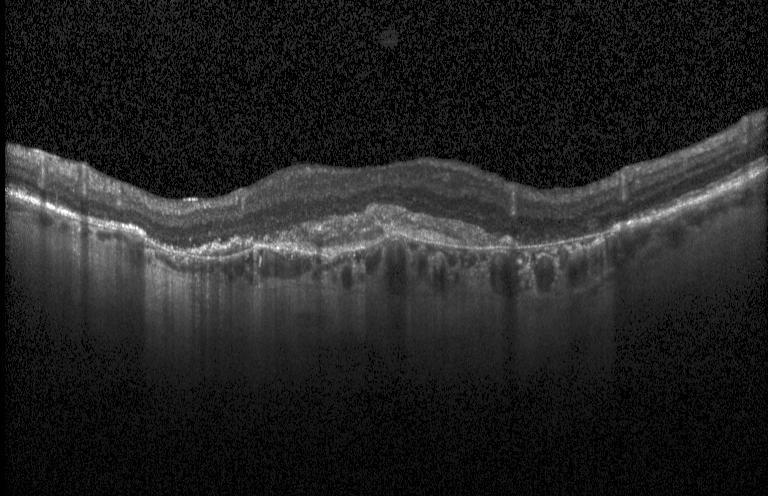 Macular OCT demonstrating a choroidal neovascular membrane.